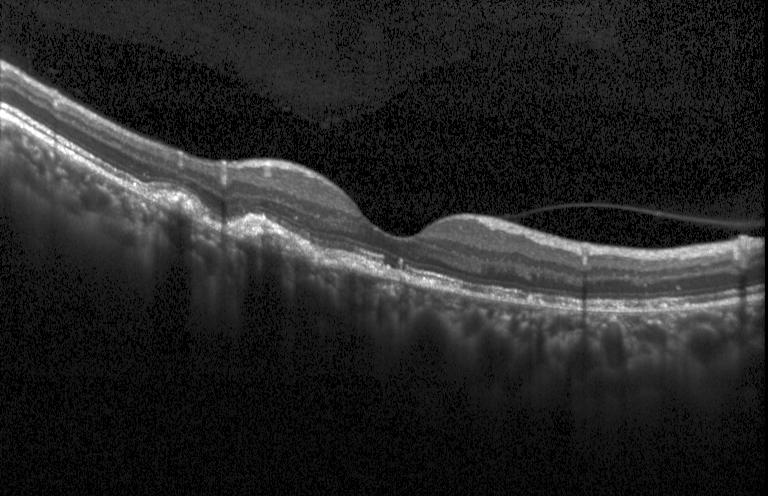 Choroidal neovascularization (CNV).